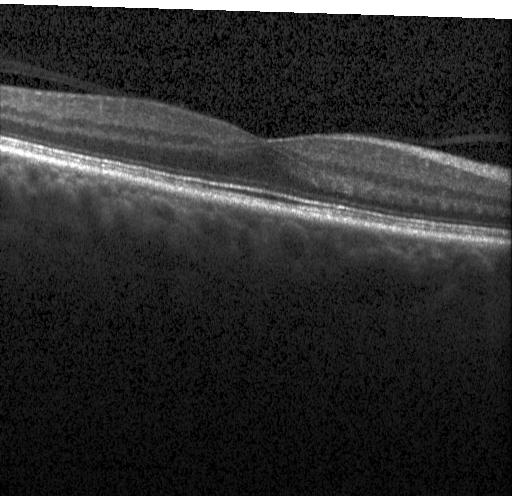
OCT line scan — Finding: no evidence of choroidal neovascularization, diabetic macular edema, or drusen.